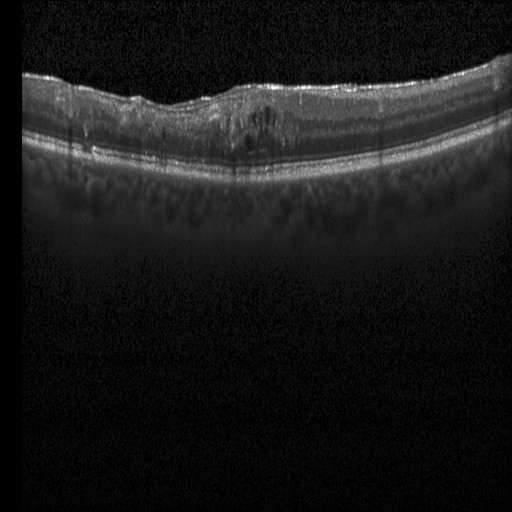 Retinal OCT cross-section showing diabetic macular edema (DME).